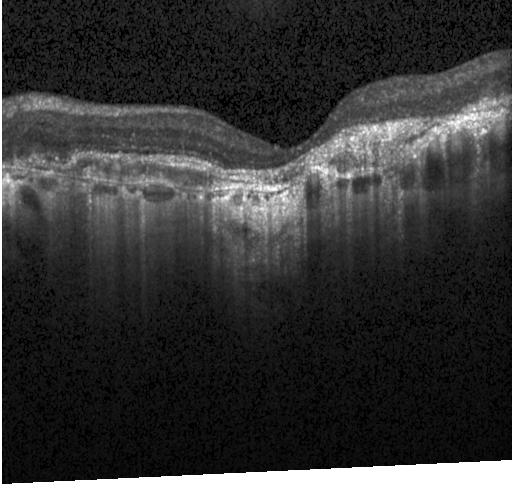
Retinal OCT B-scan.
Finding: choroidal neovascularization (CNV).